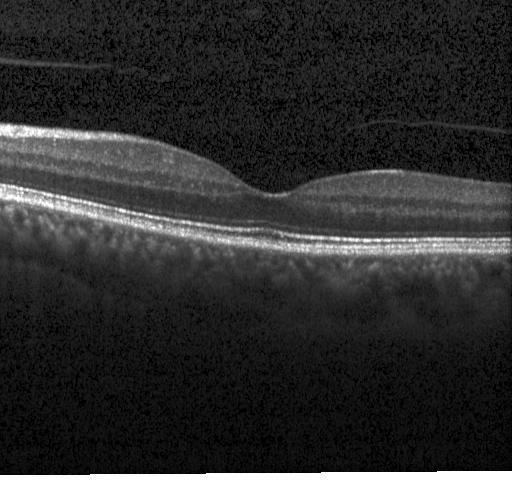
OCT finding: no CNV, no DME, and no drusen.